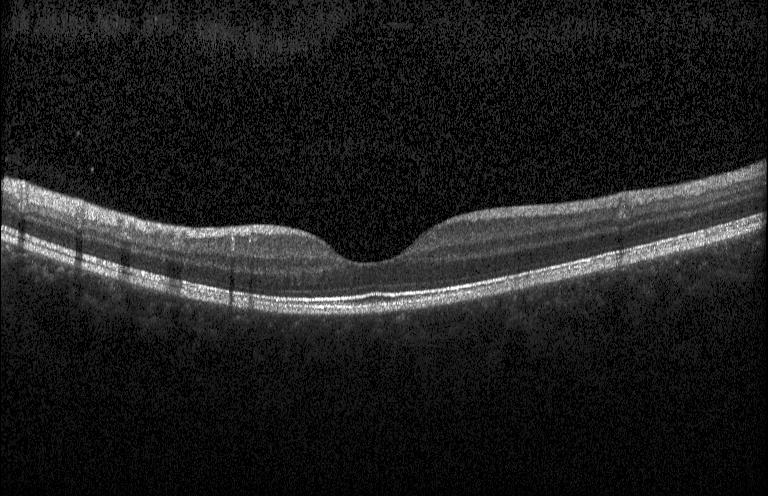

Retinal OCT cross-section
Assessment: neither choroidal neovascularization, diabetic macular edema, nor drusen.